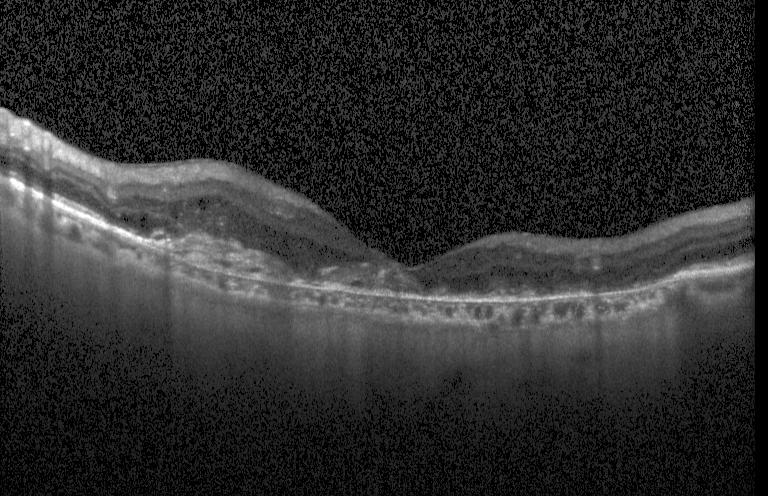

OCT line scan.
OCT finding: CNV.